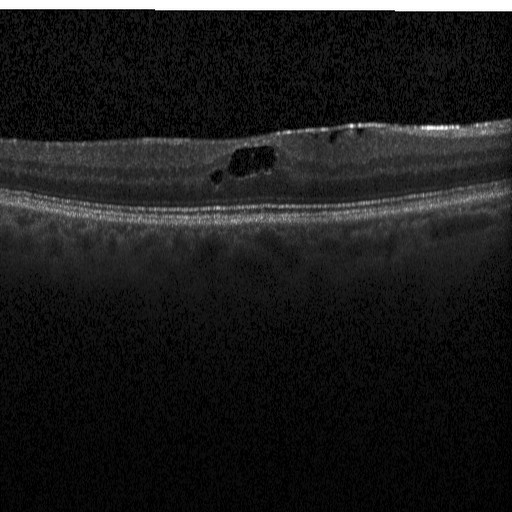
Instrument: Heidelberg Spectralis. Retinal OCT B-scan. SD-OCT. Fovea-centered. Diagnosis: DME.